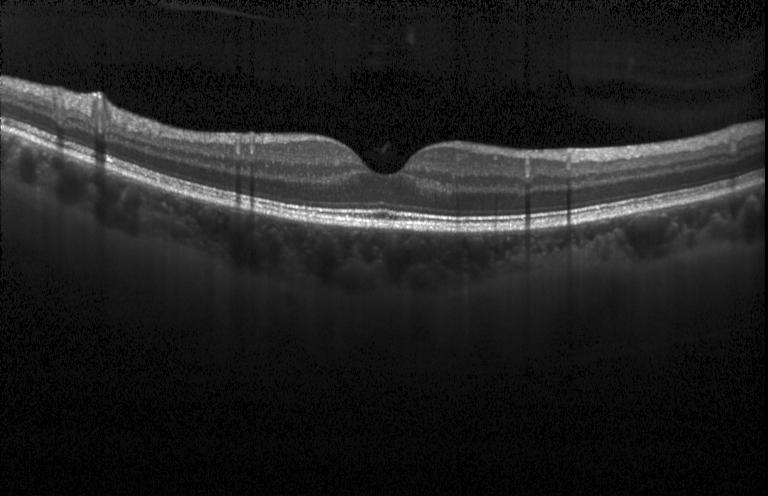
Optical coherence tomography scan; centered on the fovea; acquired on a Heidelberg Spectralis — Macular OCT: no choroidal neovascularization, no diabetic macular edema, and no drusen.